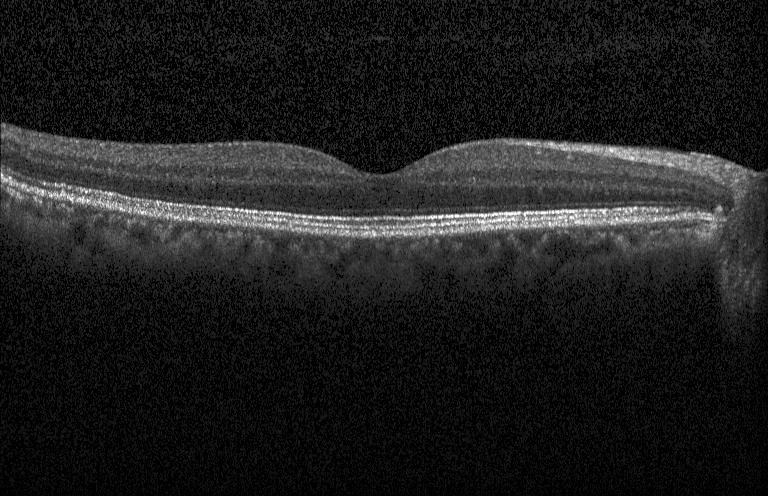

OCT scan showing no choroidal neovascularization, no diabetic macular edema, and no drusen.